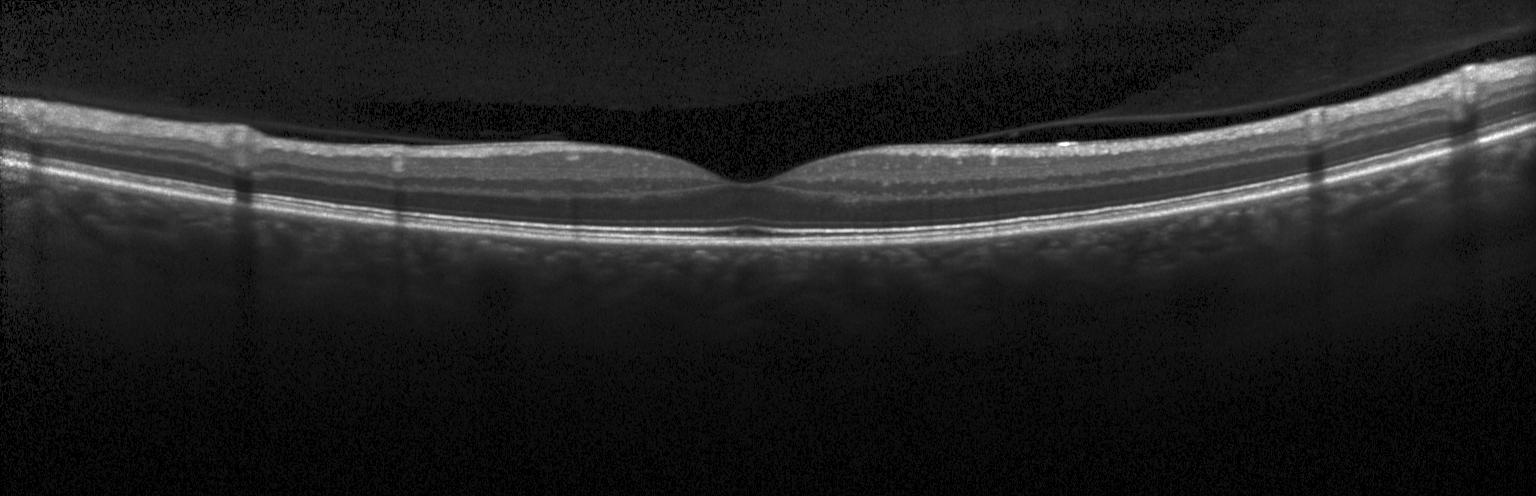
Heidelberg Spectralis OCT system, retinal OCT cross-section — Diagnosis: no choroidal neovascularization, no diabetic macular edema, and no drusen.